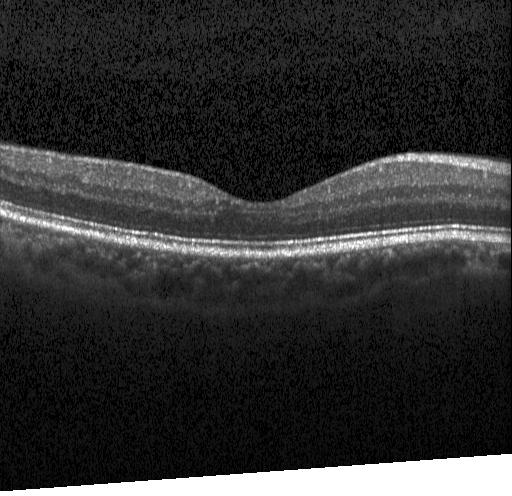 Spectral-domain OCT; optical coherence tomography scan; acquired on a Heidelberg Spectralis. Macular OCT: neither CNV, DME, nor drusen.